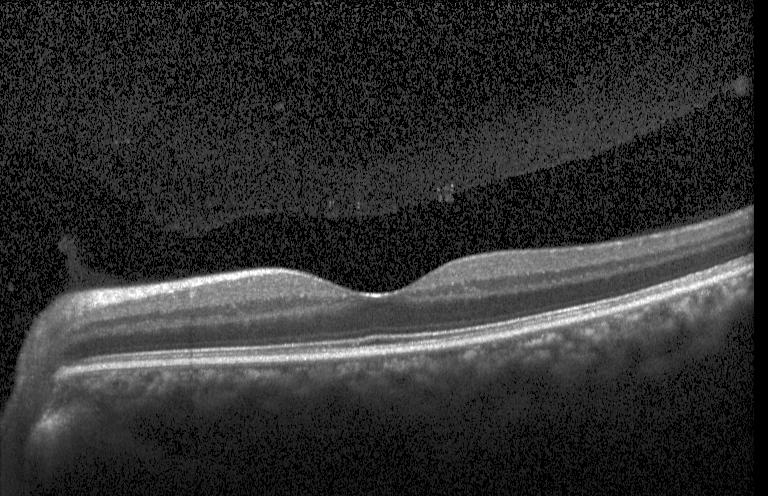 The scan shows no CNV, DME, or drusen.